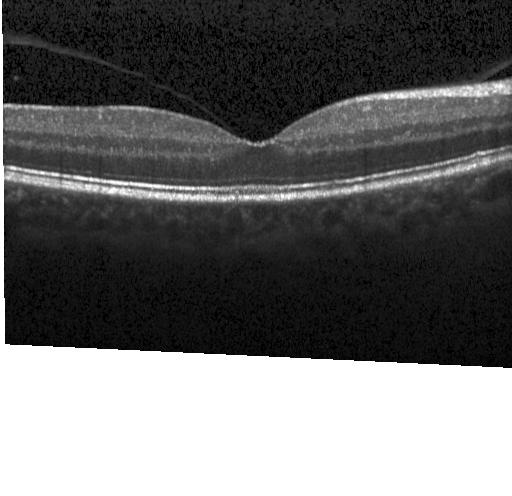
OCT line scan; macular scan; instrument: Heidelberg Spectralis.
Diagnosis: neither choroidal neovascularization, diabetic macular edema, nor drusen.